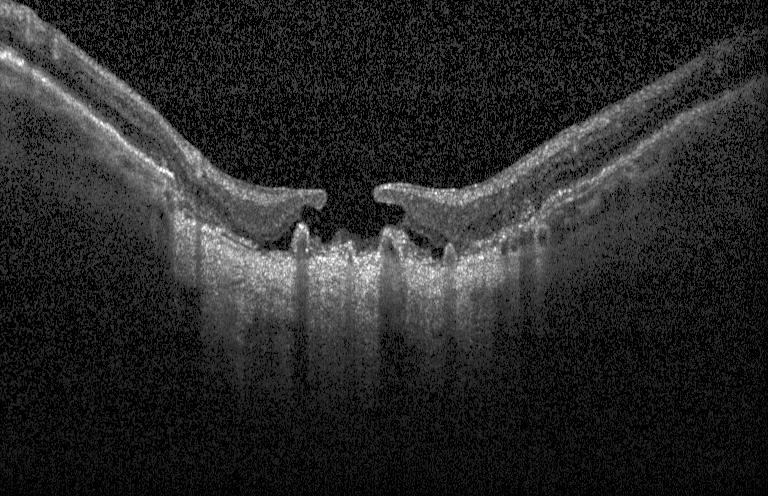 Retinal OCT cross-section showing choroidal neovascularization (CNV).